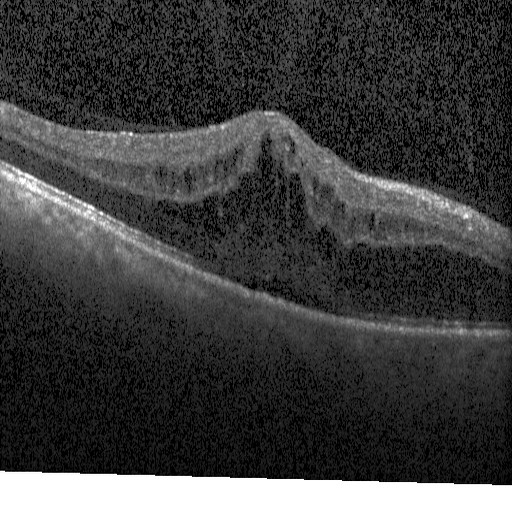
Retinal OCT cross-section showing diabetic macular edema.